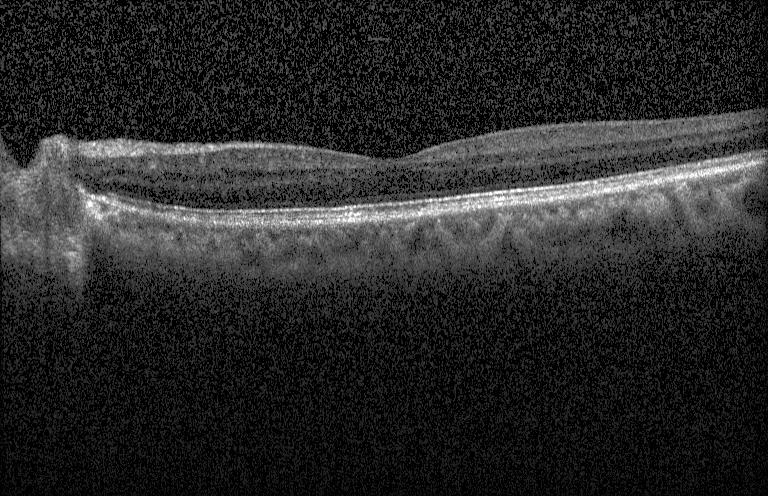 Diagnosis: no evidence of choroidal neovascularization, diabetic macular edema, or drusen.